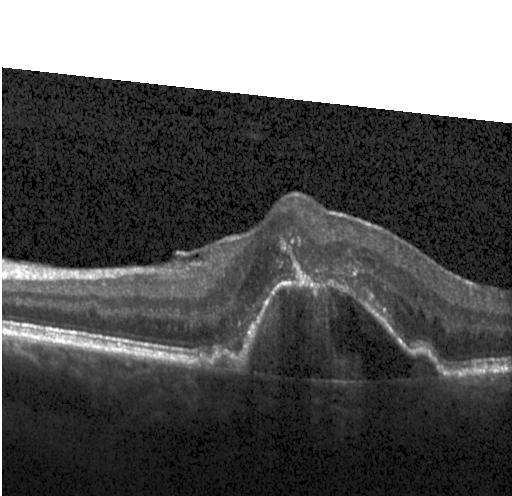 Heidelberg Spectralis, SD-OCT, optical coherence tomography B-scan, macular scan — Finding: a choroidal neovascular membrane.